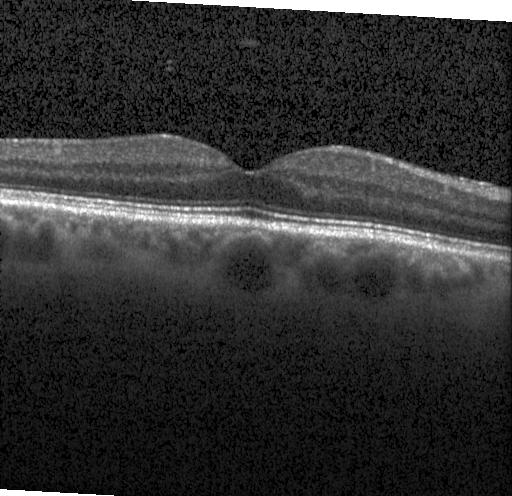 Finding: no choroidal neovascularization, diabetic macular edema, or drusen.